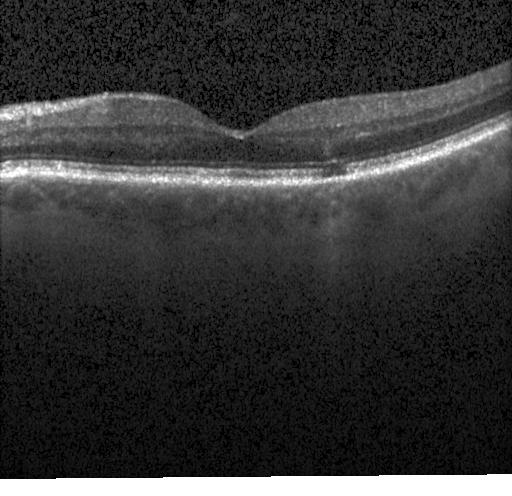
Dx: no CNV, DME, or drusen.